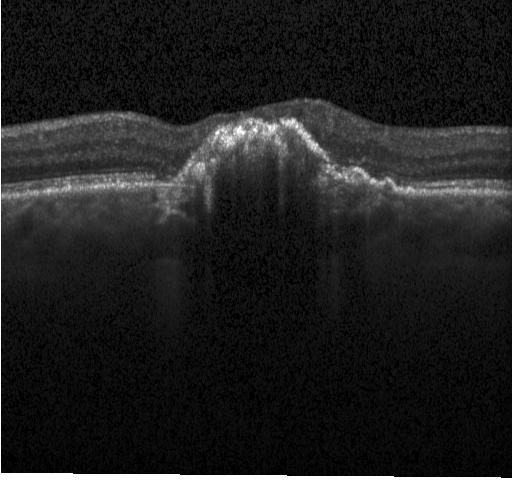 This B-scan demonstrates a choroidal neovascular membrane.